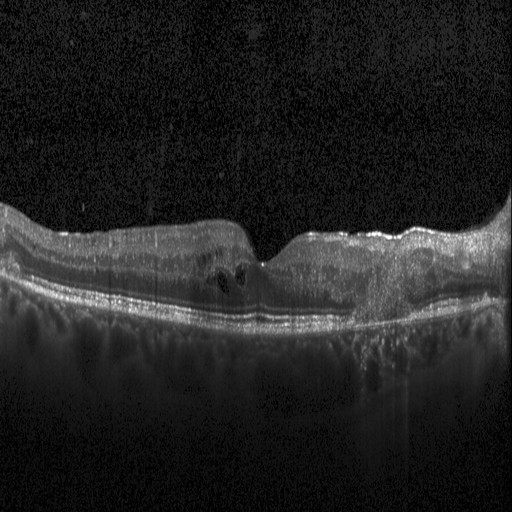
DME.